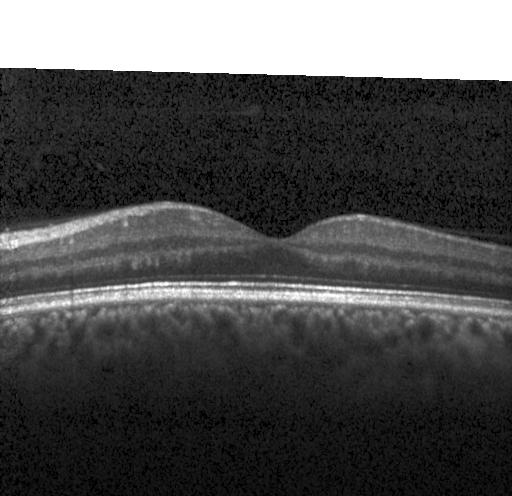
Optical coherence tomography B-scan — OCT finding: no CNV, DME, or drusen.